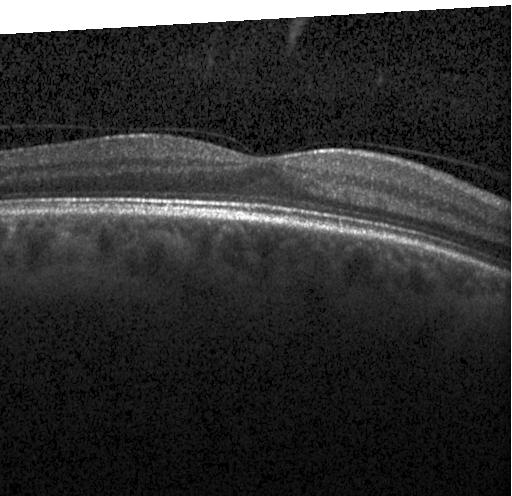
Centered on the fovea. SD-OCT. Instrument: Heidelberg Spectralis. Optical coherence tomography scan.
Diagnosis: neither CNV, DME, nor drusen.